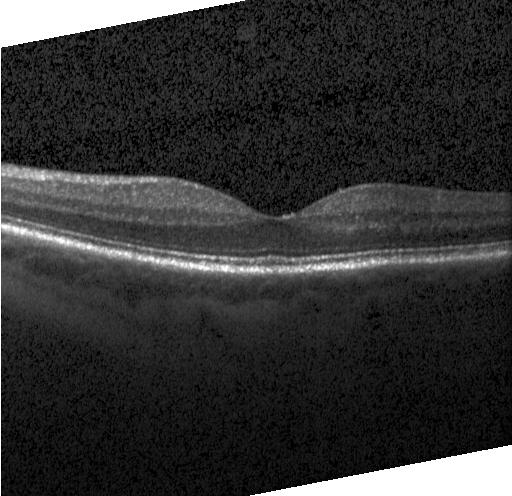

Retinal OCT B-scan · Heidelberg Spectralis OCT system — This B-scan demonstrates no evidence of CNV, DME, or drusen.